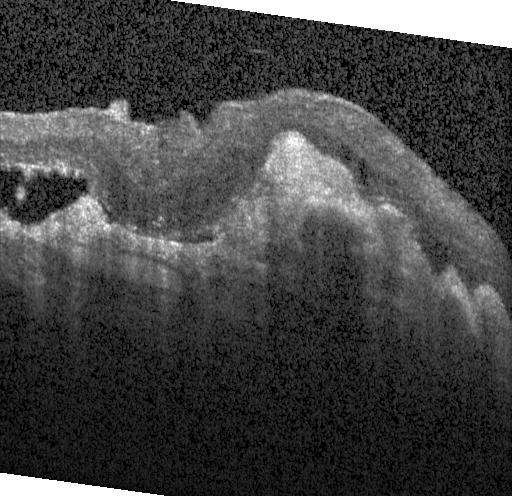

Horizontal scan through the fovea, OCT B-scan, spectral-domain OCT, instrument: Heidelberg Spectralis. Assessment: choroidal neovascularization (CNV).